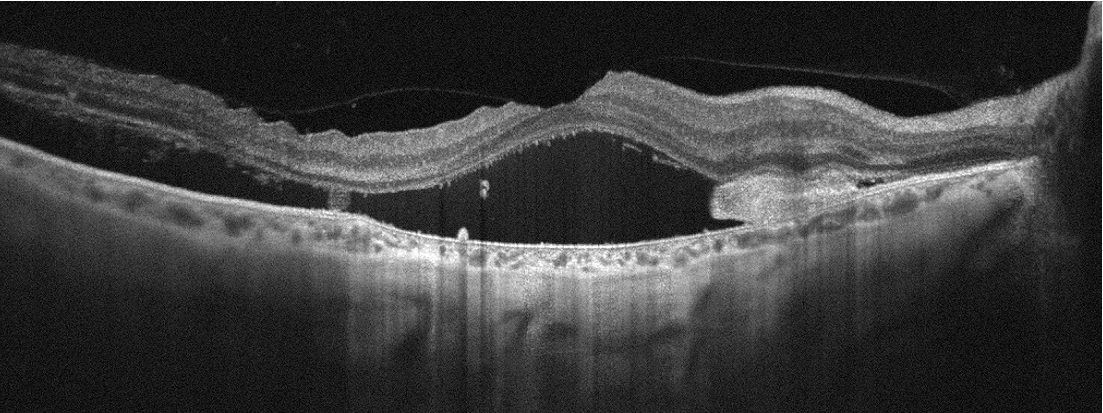 Optical coherence tomography B-scan. Dx: age-related macular degeneration (AMD).